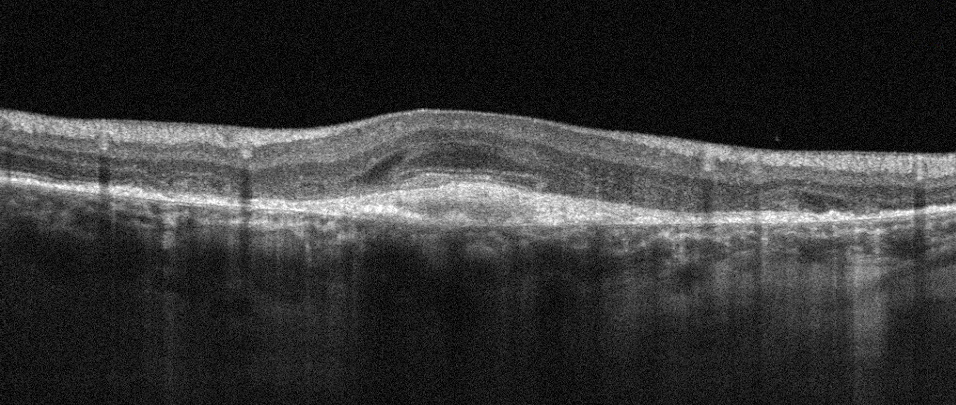
Optical coherence tomography B-scan, instrument: Optovue Avanti RTVue XR
Impression: age-related macular degeneration (AMD).